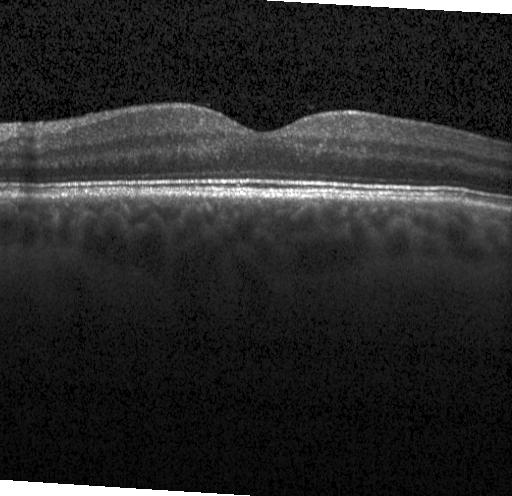 Finding: no CNV, no DME, and no drusen.